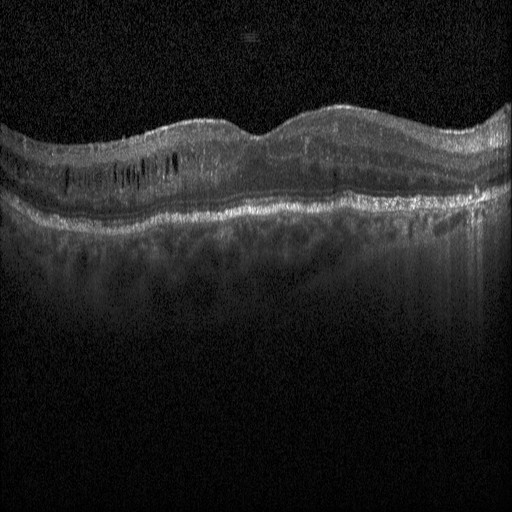 SD-OCT. Optical coherence tomography B-scan. Fovea-centered
Impression: DME.